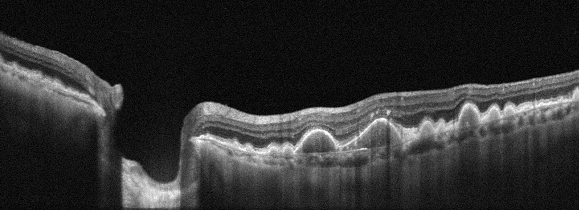 Optical coherence tomography B-scan, macular scan, Optovue Avanti RTVue XR
The scan shows age-related macular degeneration (AMD).